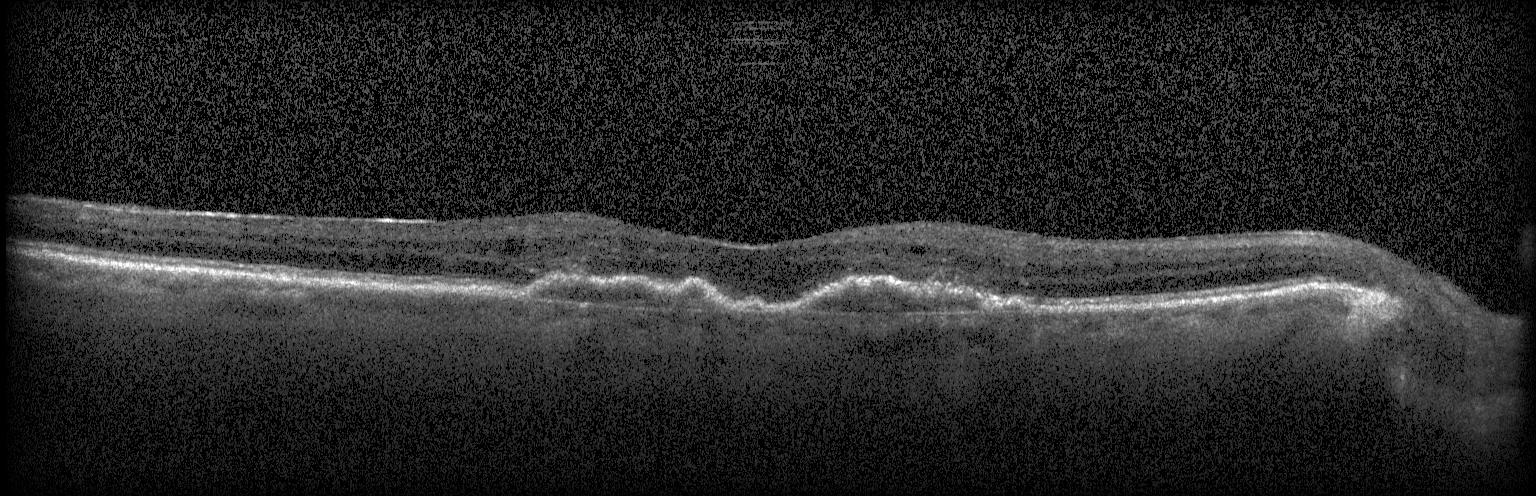
SD-OCT · macular scan · OCT B-scan · acquired on a Heidelberg Spectralis.
Dx: choroidal neovascularization.